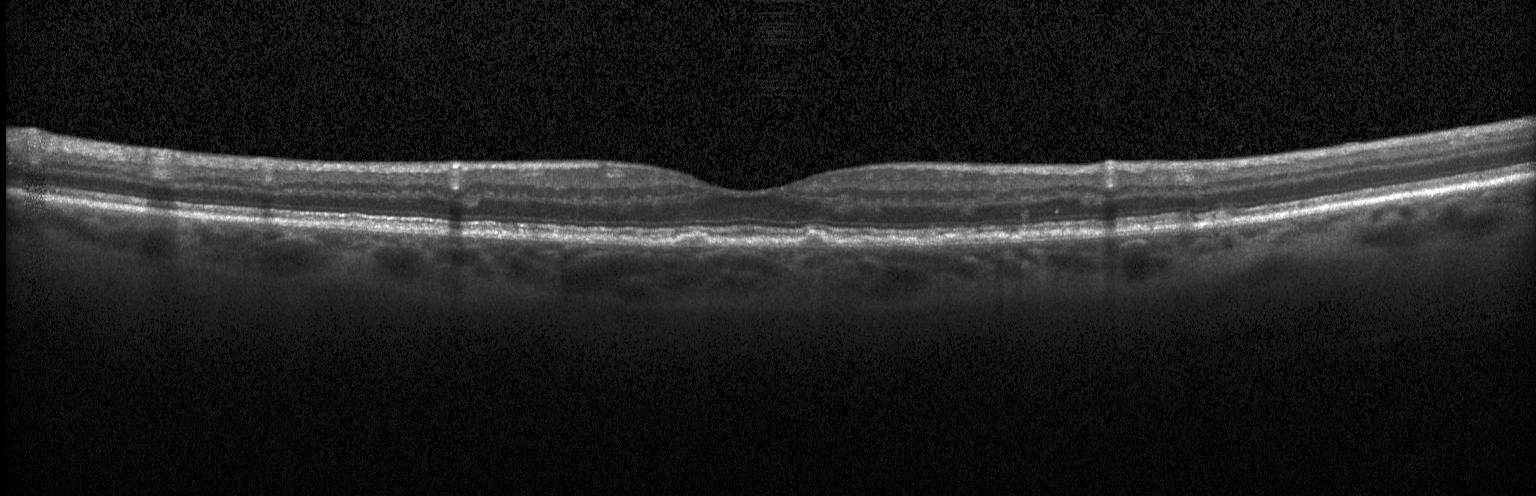 OCT line scan. The scan shows sub-RPE drusenoid deposits.